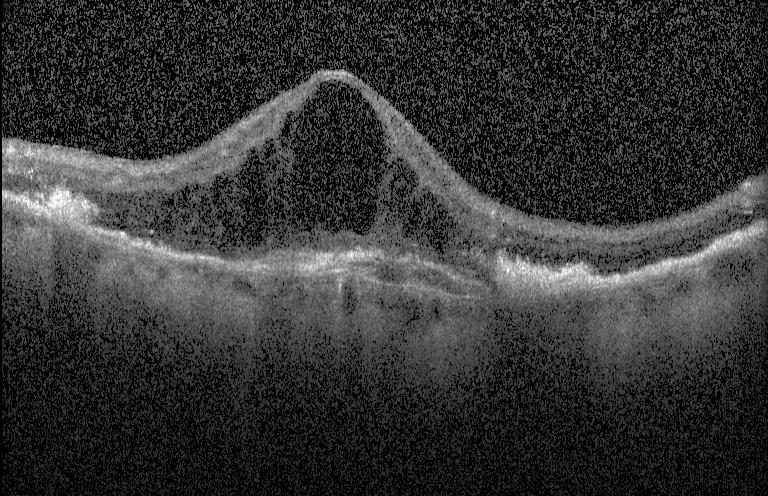 Heidelberg Spectralis. OCT line scan. Spectral-domain optical coherence tomography. Centered on the fovea.
This B-scan demonstrates choroidal neovascularization (CNV).